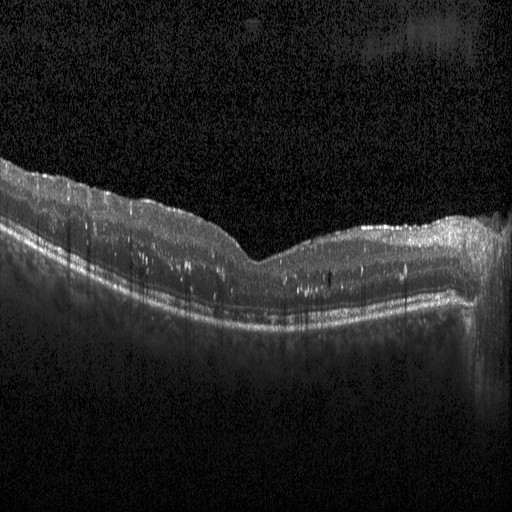

Through the macula · instrument: Heidelberg Spectralis · OCT B-scan · spectral-domain OCT.
Diagnosis: diabetic macular edema.